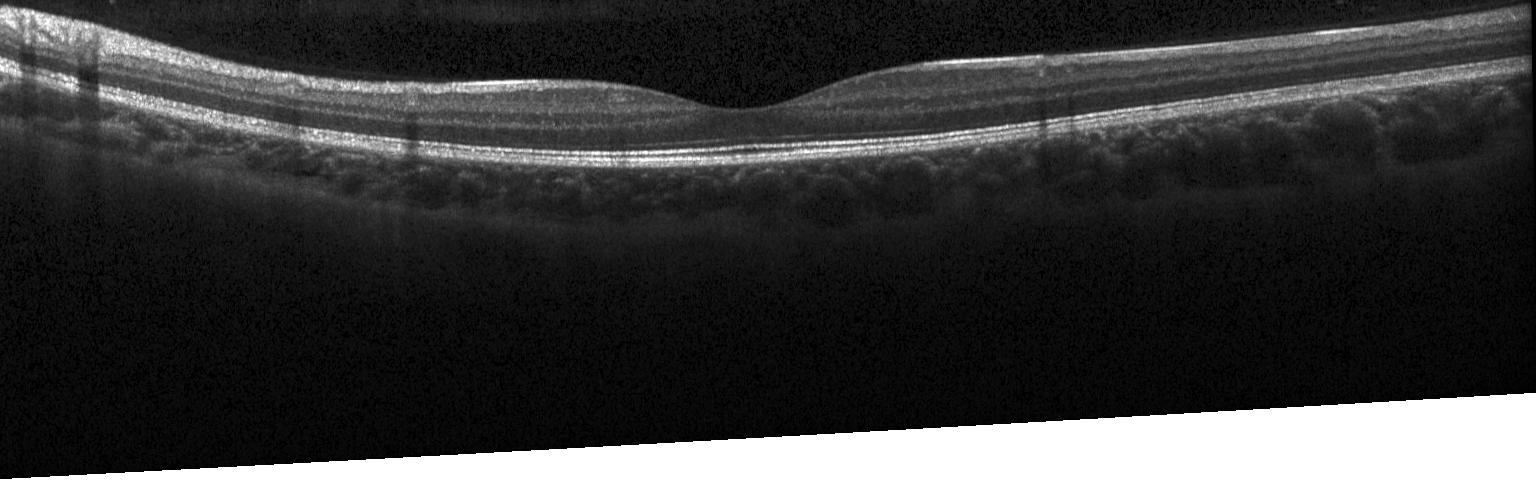

Optical coherence tomography scan; Heidelberg Spectralis; through the macula
The scan shows no evidence of CNV, DME, or drusen.